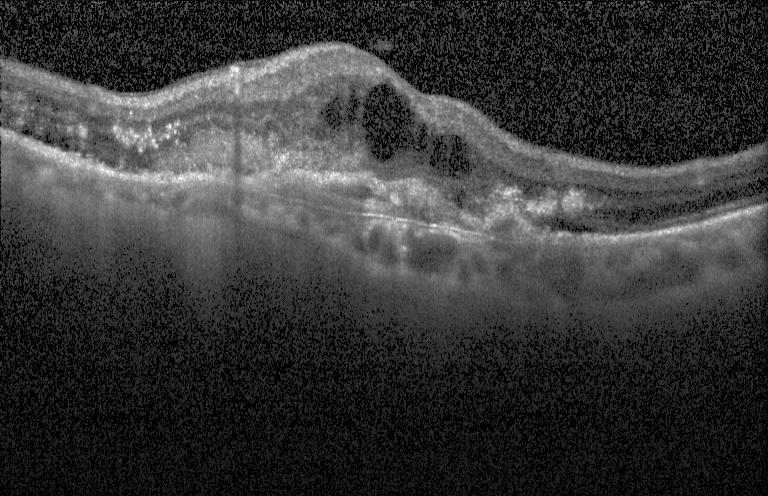 Retinal OCT B-scan; spectral-domain OCT; instrument: Heidelberg Spectralis; centered on the fovea.
Finding: choroidal neovascularization (CNV).